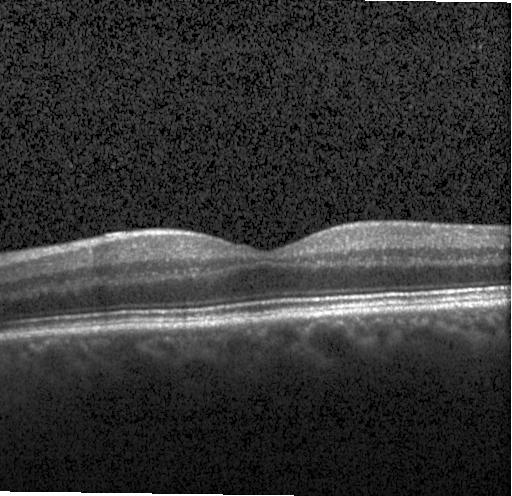

Macular OCT demonstrating neither CNV, DME, nor drusen.